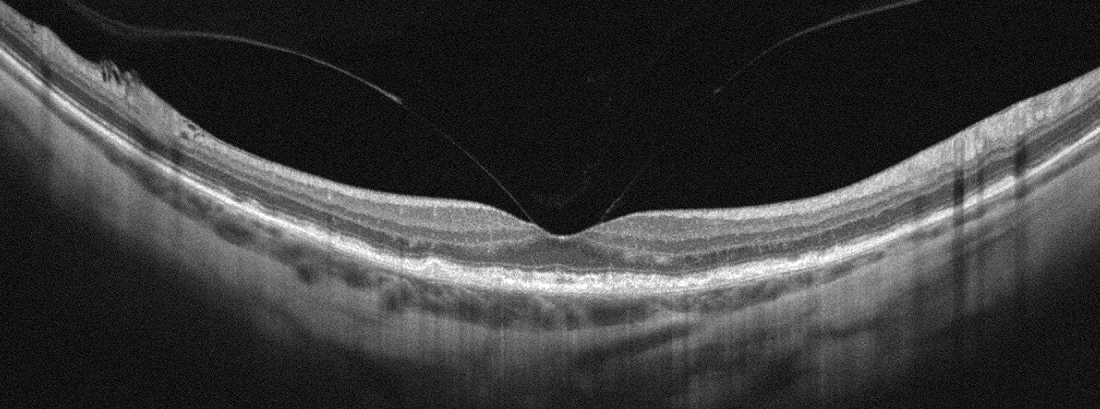
Macular scan, OCT B-scan. Finding: AMD.